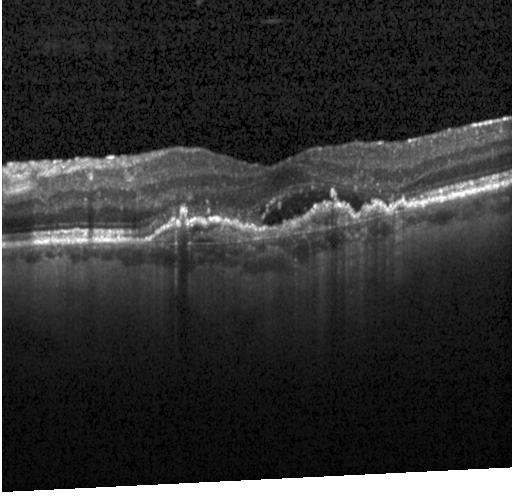 OCT line scan; spectral-domain OCT; through the macula — CNV.